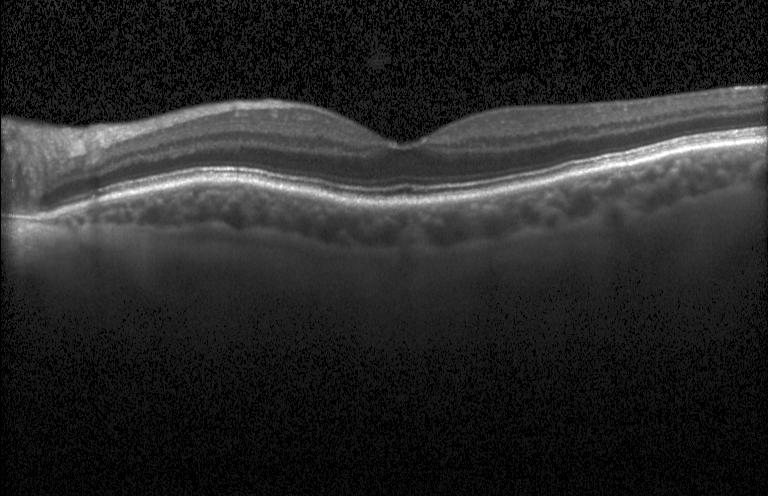

OCT B-scan
Diagnosis: no evidence of CNV, DME, or drusen.